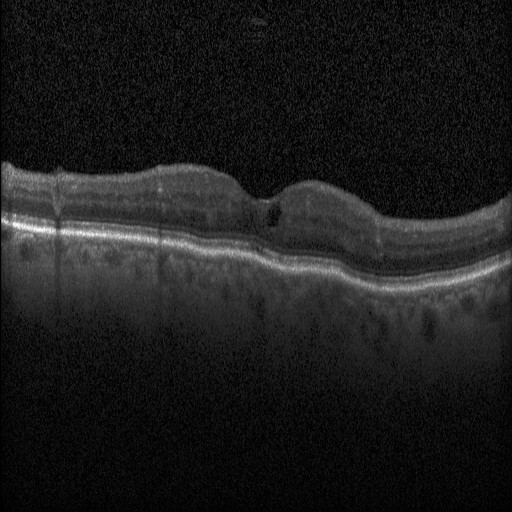 Heidelberg Spectralis, fovea-centered, optical coherence tomography scan, spectral-domain OCT — Impression: diabetic macular edema.